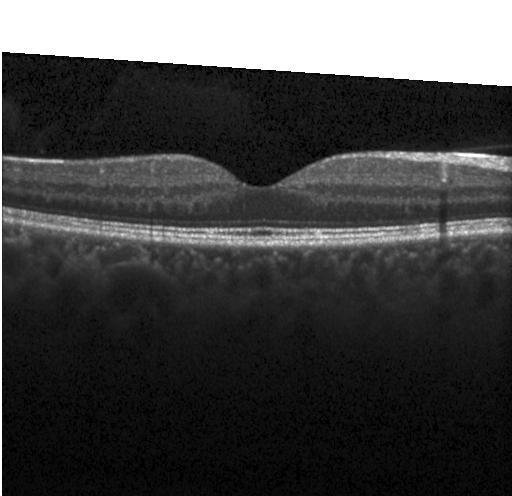
Finding: no CNV, no DME, and no drusen.